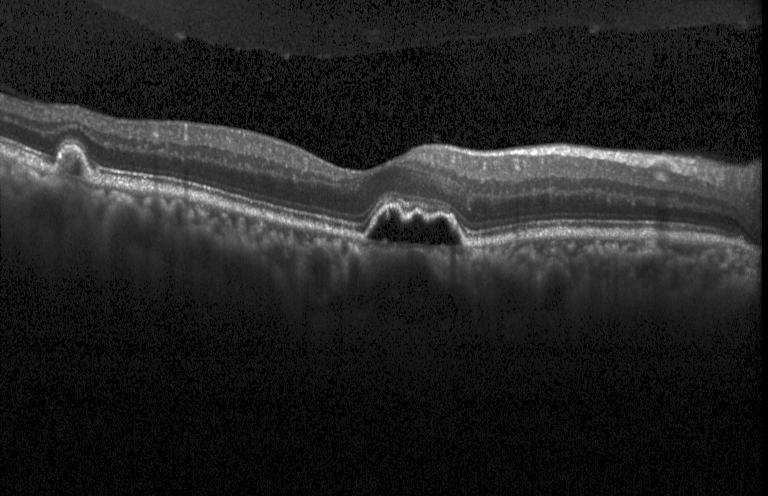 Spectral-domain optical coherence tomography, OCT B-scan
Finding: choroidal neovascularization (CNV).